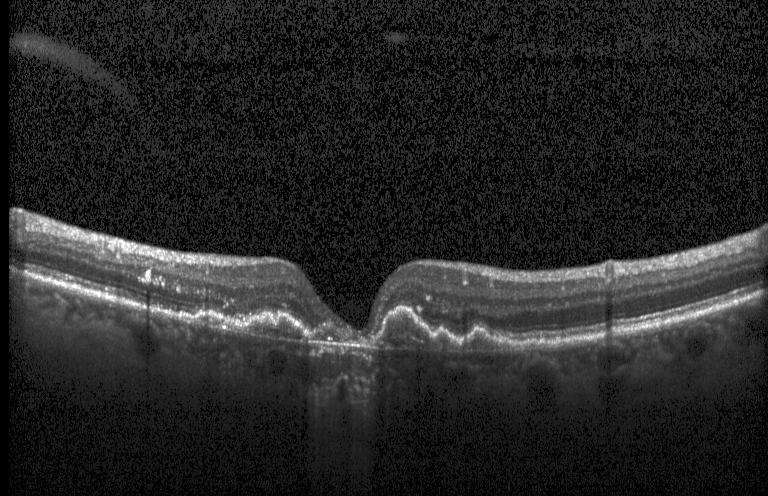

Acquired on a Heidelberg Spectralis. OCT B-scan. SD-OCT.
Diagnosis: choroidal neovascularization.